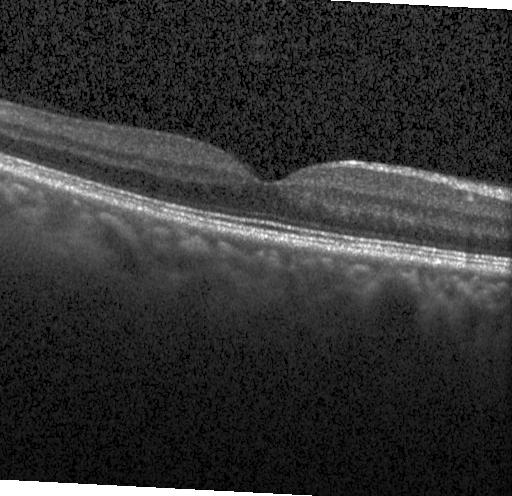
Heidelberg Spectralis OCT system · retinal OCT B-scan — Finding: no choroidal neovascularization, diabetic macular edema, or drusen.